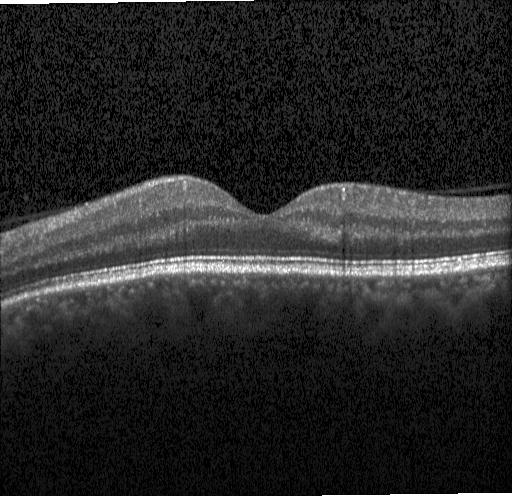 Through the macula, optical coherence tomography B-scan — Macular OCT: neither CNV, DME, nor drusen.